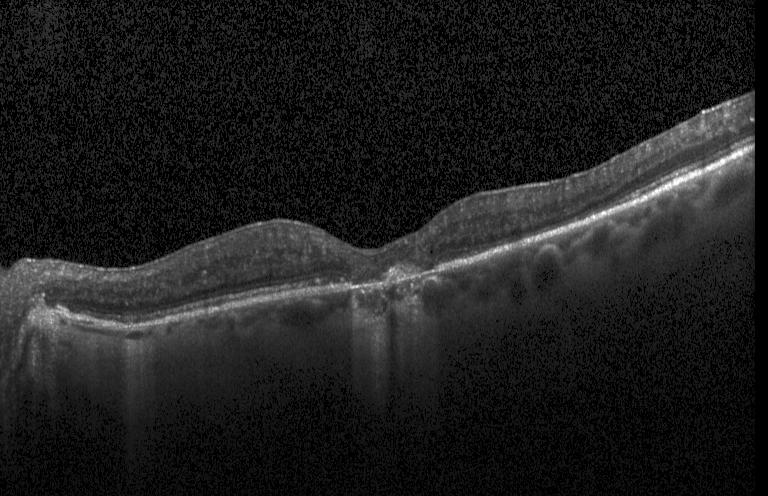 This B-scan demonstrates choroidal neovascularization (CNV).